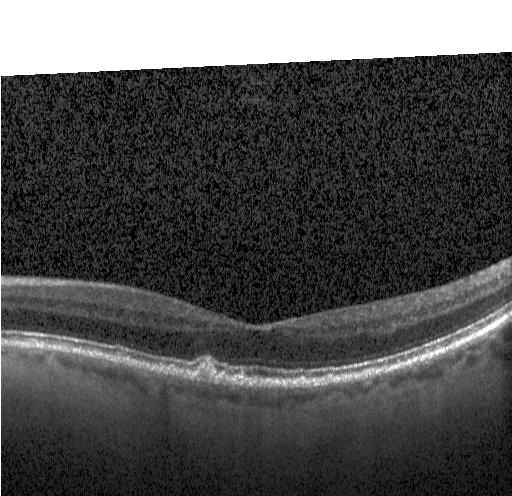

Optical coherence tomography scan. This B-scan demonstrates sub-RPE drusenoid deposits.